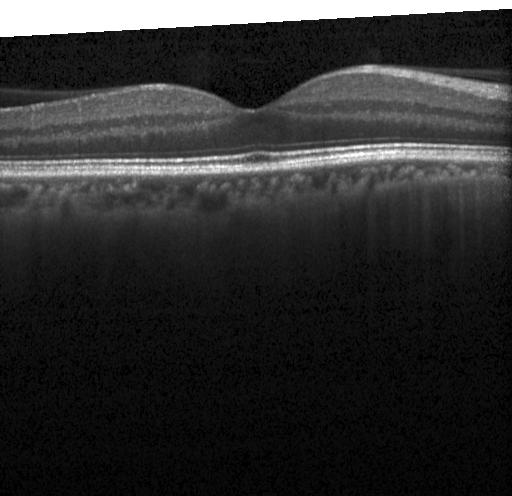

This B-scan demonstrates neither CNV, DME, nor drusen.